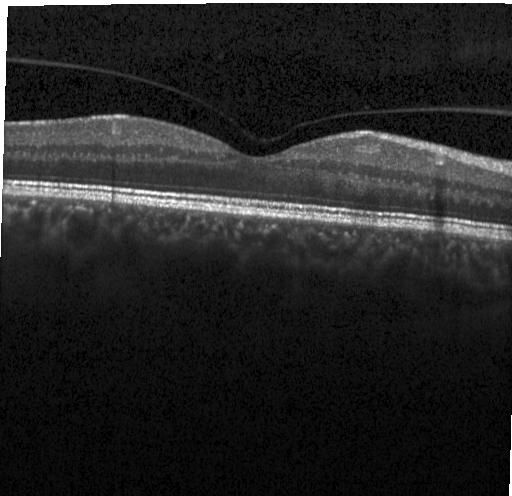
Assessment: no evidence of choroidal neovascularization, diabetic macular edema, or drusen.